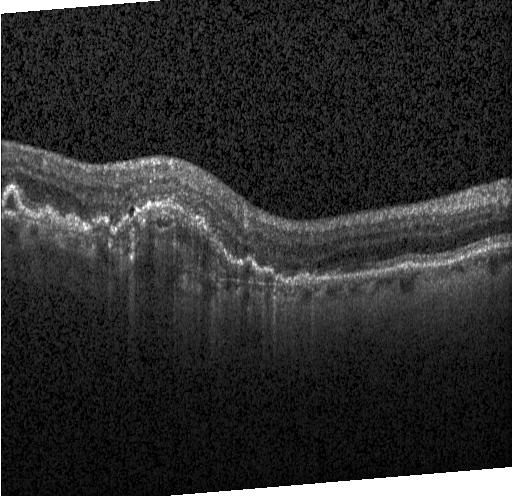
Retinal OCT cross-section showing CNV.